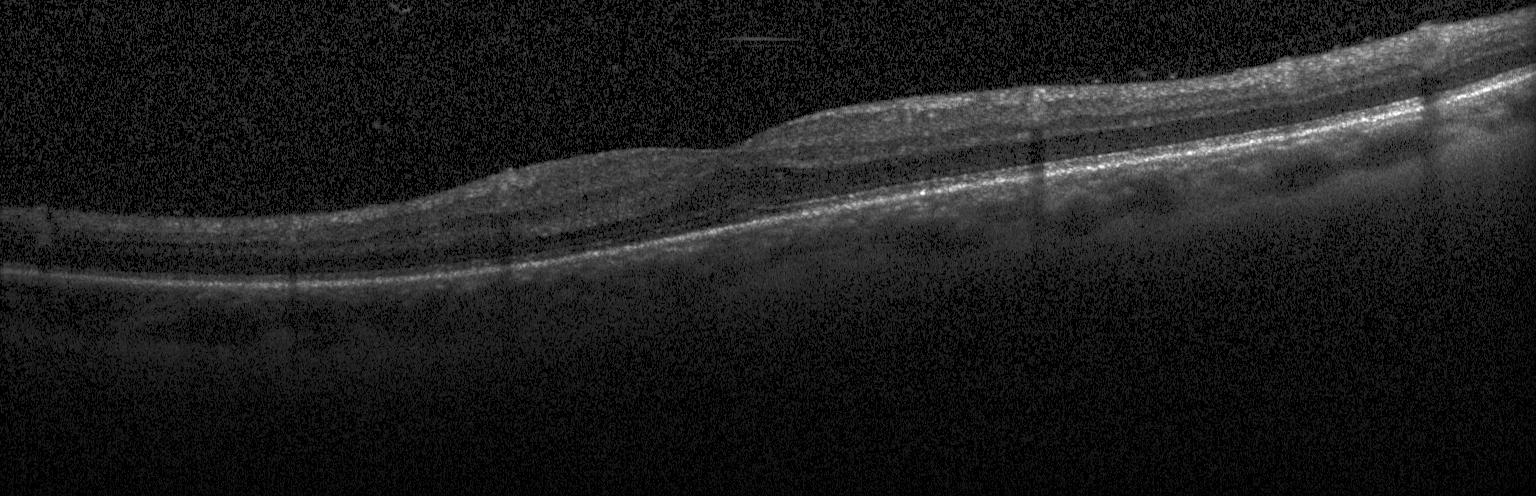 Instrument: Heidelberg Spectralis; through the macula; OCT B-scan; spectral-domain OCT. Dx: no CNV, no DME, and no drusen.